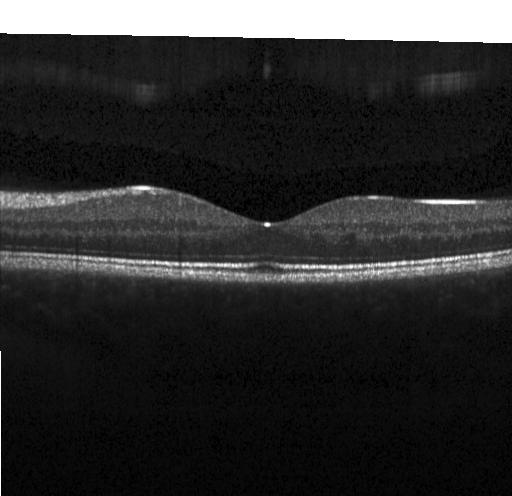 OCT B-scan.
Finding: no CNV, DME, or drusen.